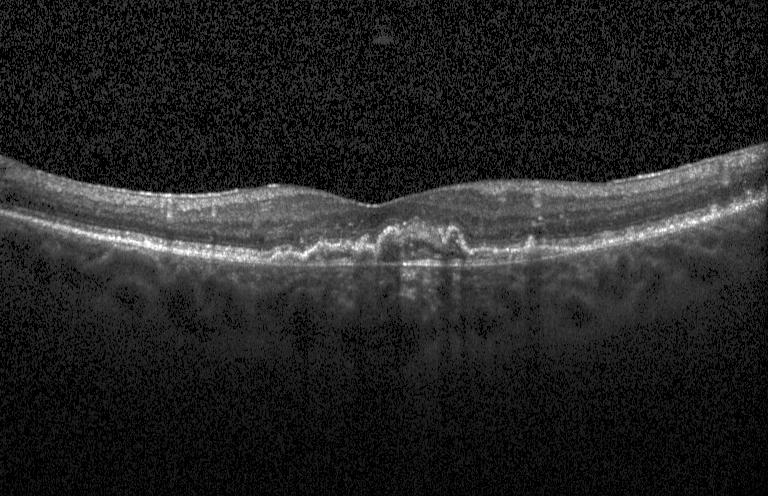 The scan shows CNV.